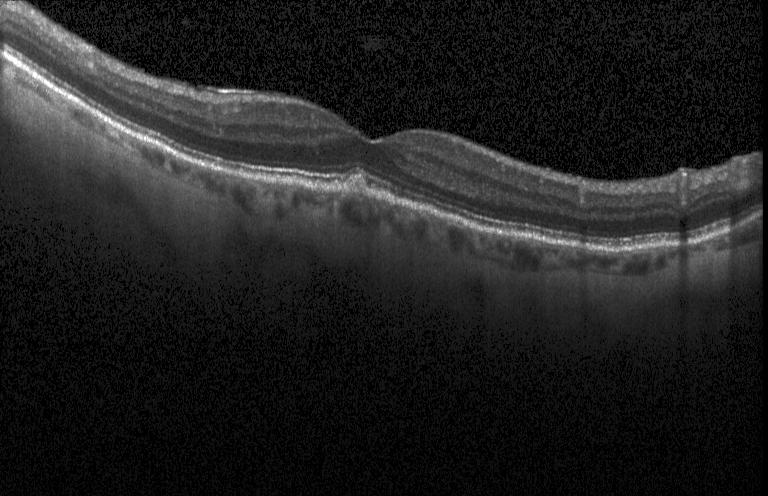 Instrument: Heidelberg Spectralis, OCT line scan — Macular OCT: multiple drusen.